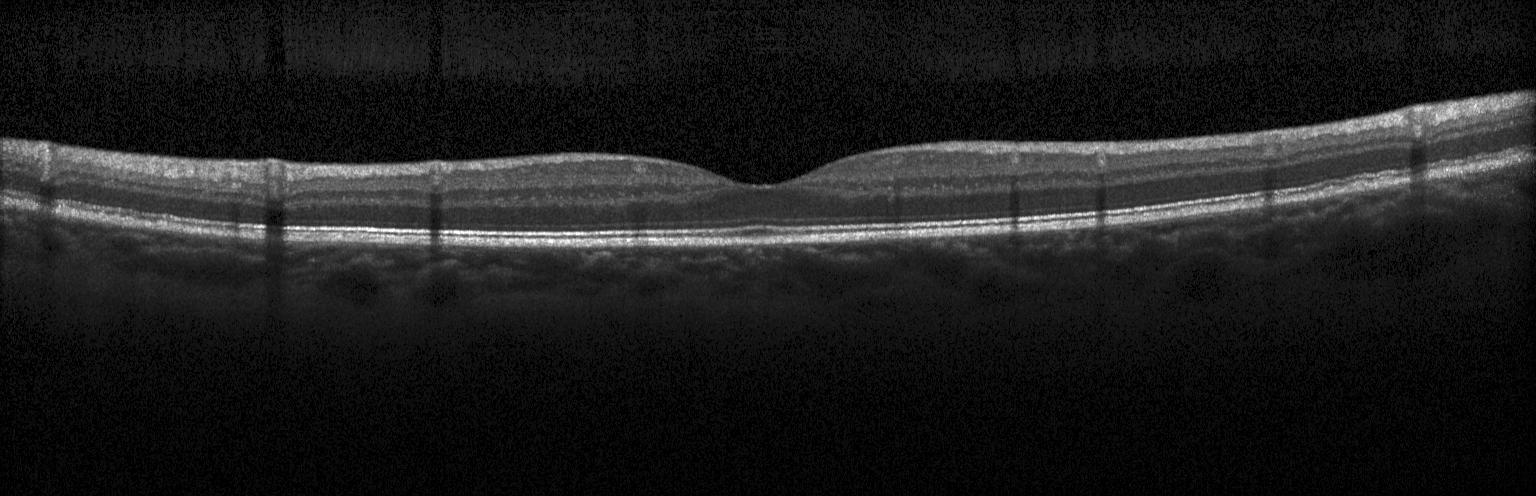

Spectral-domain optical coherence tomography, optical coherence tomography B-scan, horizontal scan through the fovea, acquired on a Heidelberg Spectralis. The scan shows no choroidal neovascularization, diabetic macular edema, or drusen.